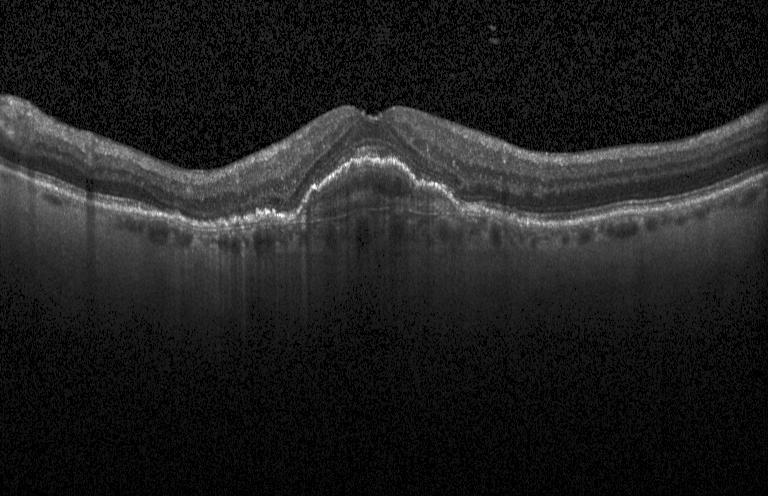

Optical coherence tomography B-scan. Spectral-domain OCT — Assessment: choroidal neovascularization (CNV).